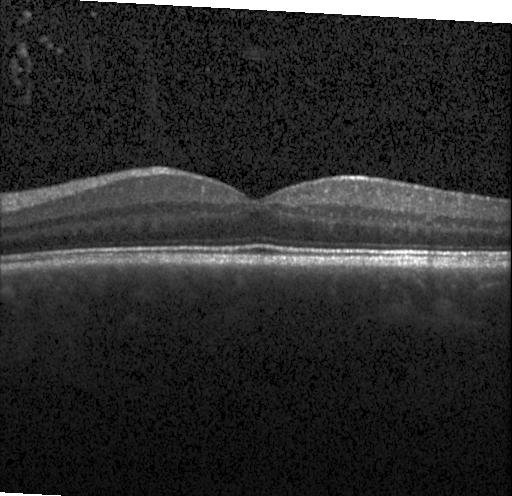 OCT line scan — Impression: no evidence of choroidal neovascularization, diabetic macular edema, or drusen.